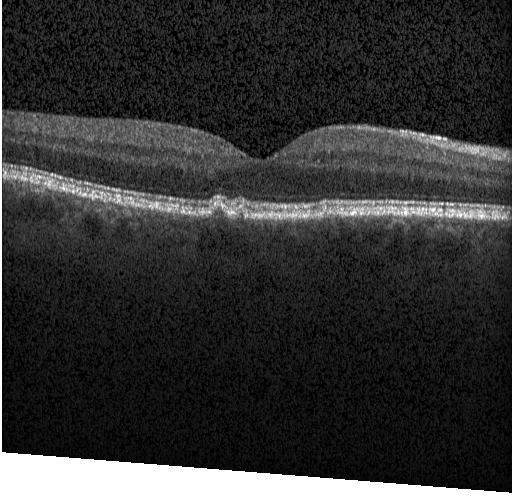
Retinal OCT B-scan · acquired on a Heidelberg Spectralis.
Impression: sub-RPE drusenoid deposits.